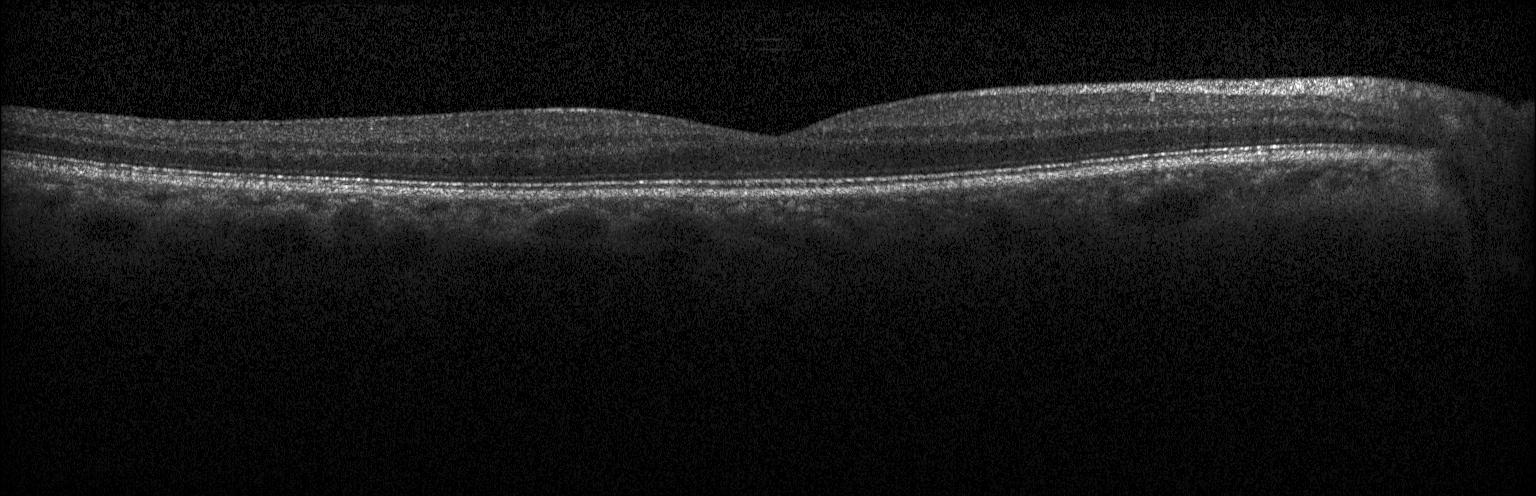 Diagnosis: no choroidal neovascularization, diabetic macular edema, or drusen.